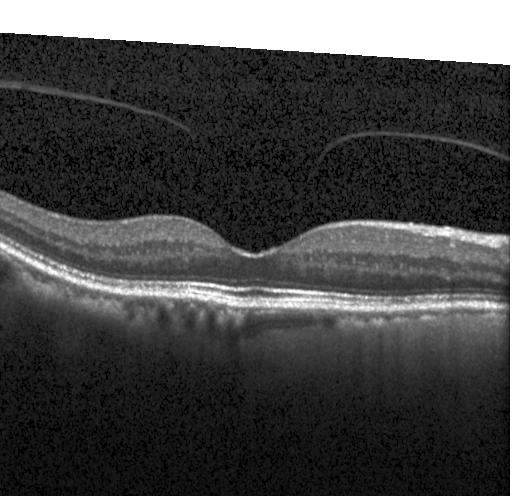 Optical coherence tomography B-scan; macular scan; spectral-domain OCT; Heidelberg Spectralis.
Macular OCT: no evidence of CNV, DME, or drusen.